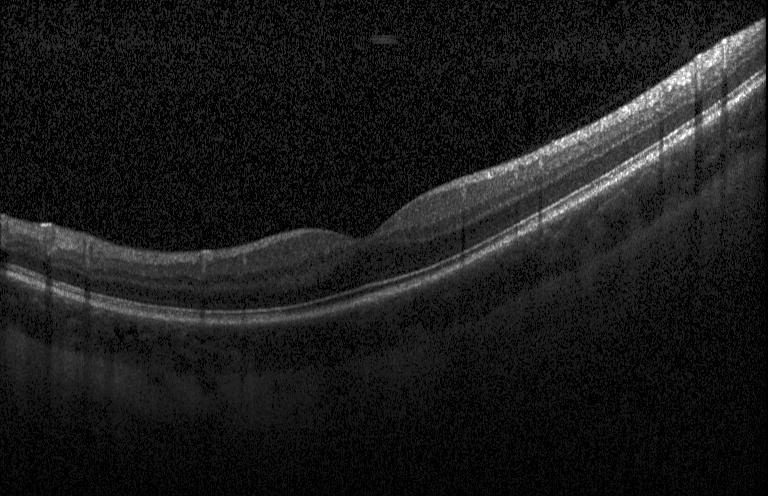 Assessment: no evidence of choroidal neovascularization, diabetic macular edema, or drusen.